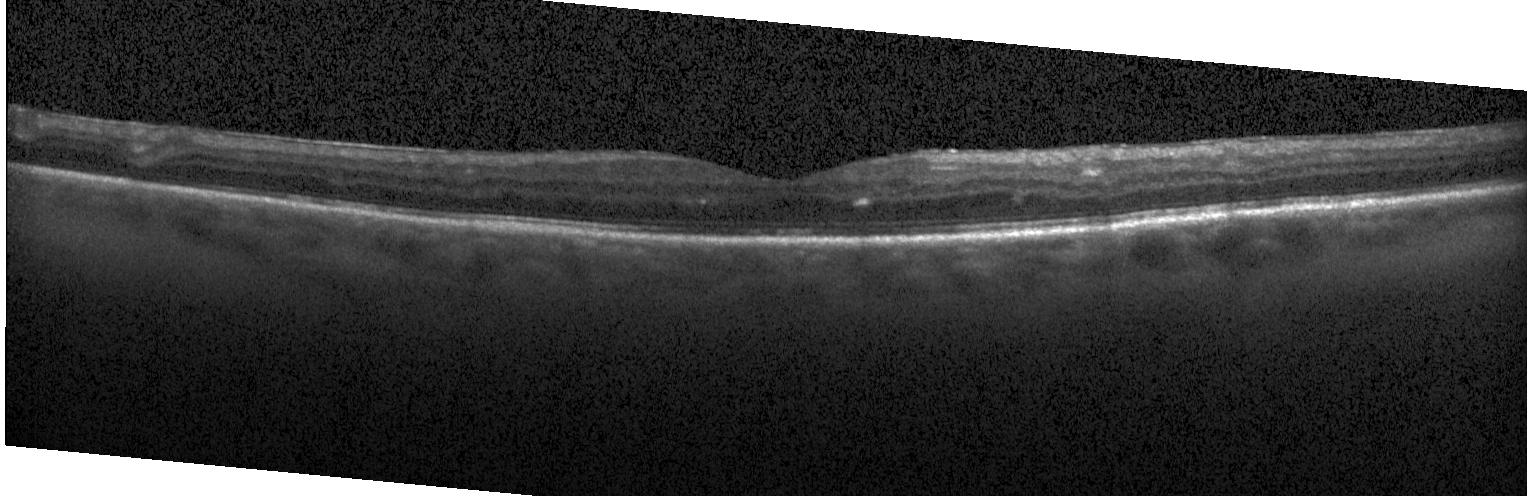

Optical coherence tomography B-scan; fovea-centered; Heidelberg Spectralis OCT system
Finding: no choroidal neovascularization, diabetic macular edema, or drusen.